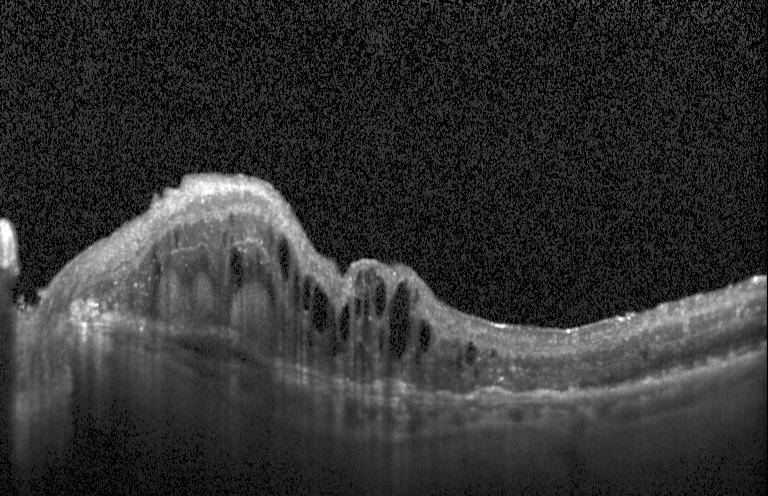 Through the macula, Heidelberg Spectralis OCT system, spectral-domain optical coherence tomography, OCT B-scan. Assessment: CNV.